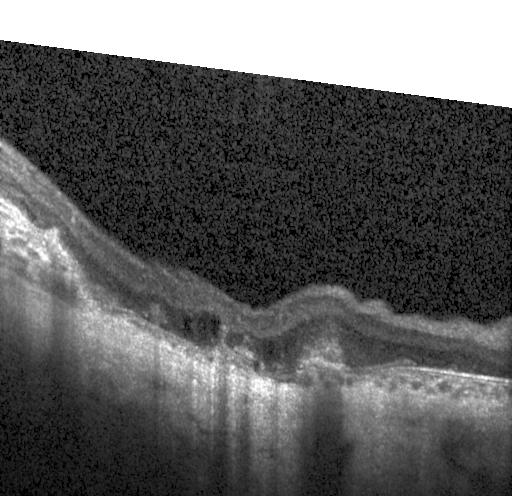
Finding: a choroidal neovascular membrane.